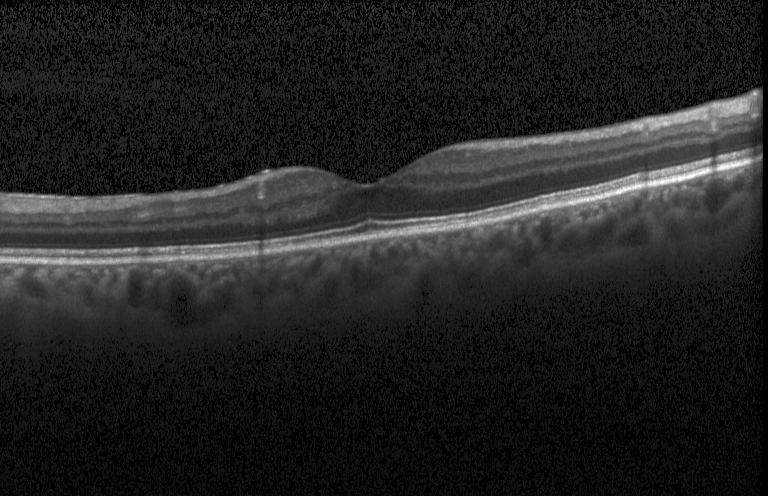 This B-scan demonstrates no choroidal neovascularization, diabetic macular edema, or drusen.